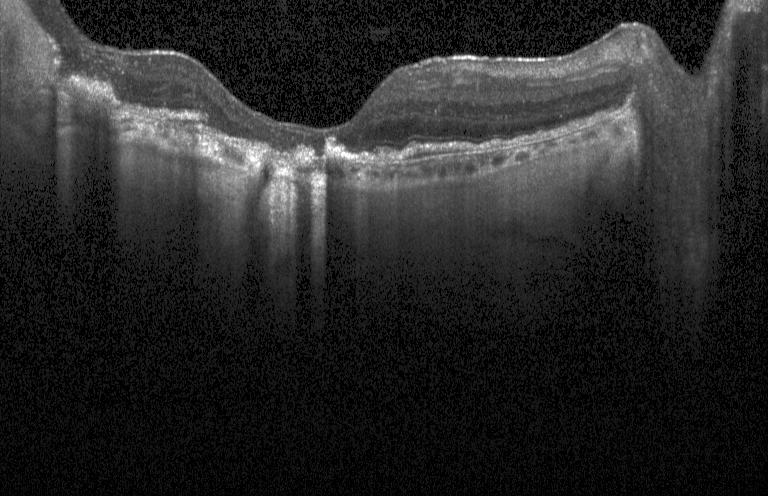

OCT B-scan showing choroidal neovascularization.